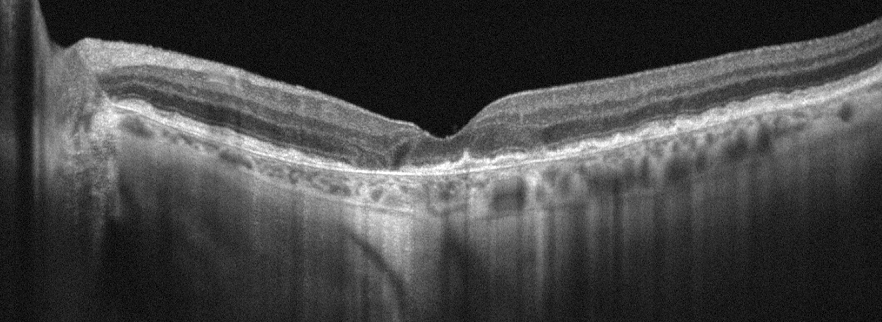 Retinal OCT cross-section · instrument: Optovue Avanti RTVue XR · oculus sinister · through the macula — Diagnosis: age-related macular degeneration.